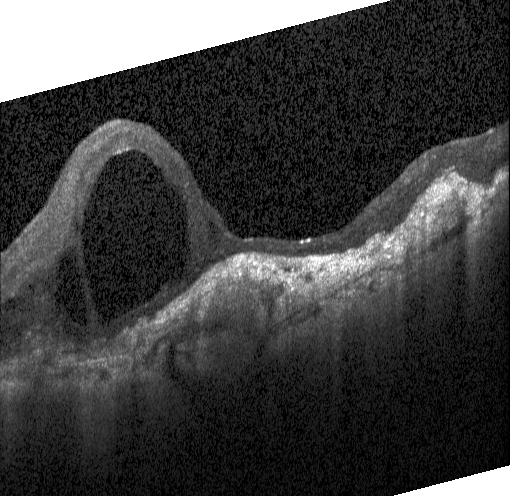 Retinal OCT cross-section, acquired on a Heidelberg Spectralis, SD-OCT, macular scan — Assessment: choroidal neovascularization.